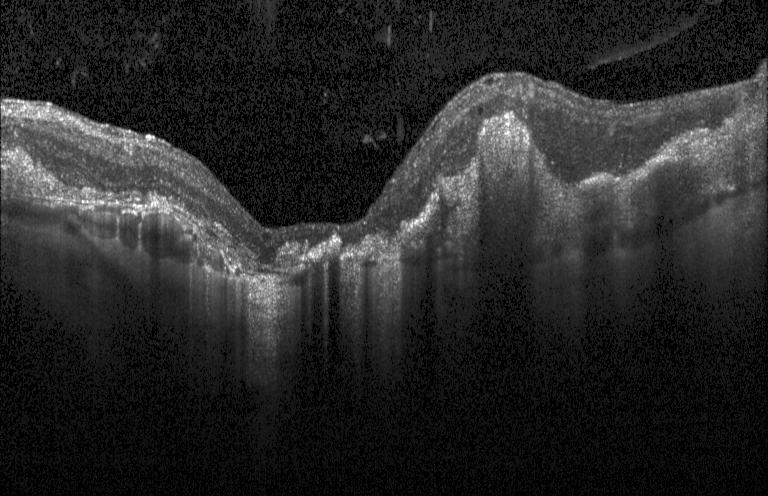 Macular OCT: a choroidal neovascular membrane.